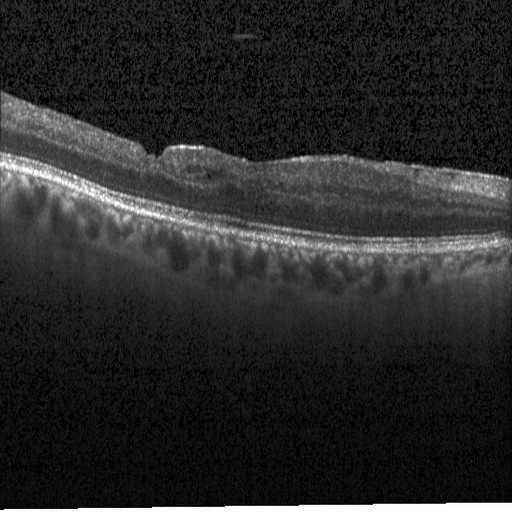
Acquired on a Heidelberg Spectralis; retinal OCT cross-section; through the macula.
Diagnosis: DME.